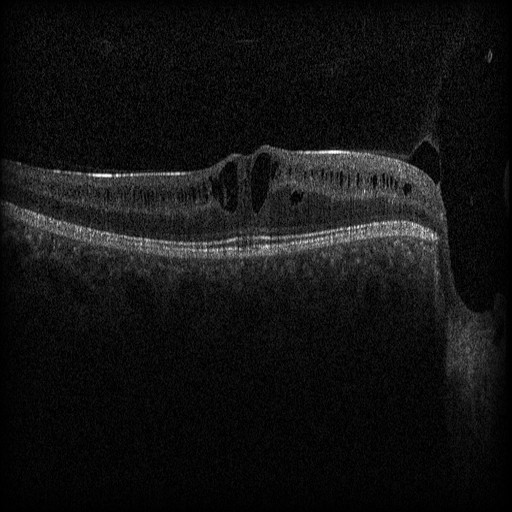
Spectral-domain OCT B-scan: DME.